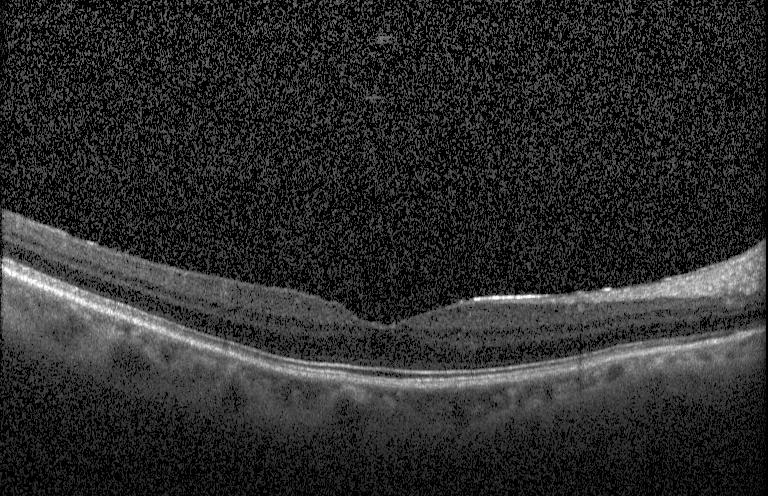
Macular OCT: no CNV, no DME, and no drusen.